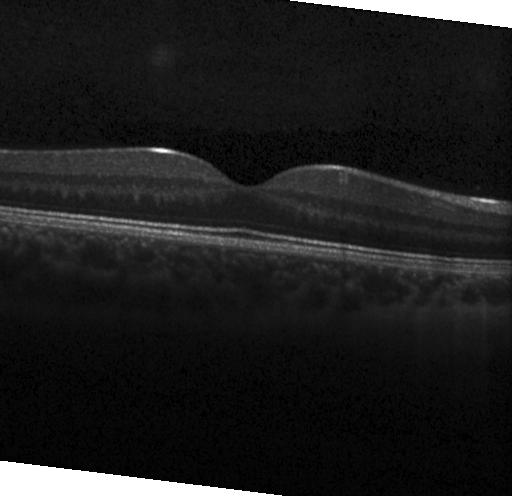

Spectral-domain optical coherence tomography · optical coherence tomography scan · through the macula · Heidelberg Spectralis OCT system. Impression: no CNV, no DME, and no drusen.